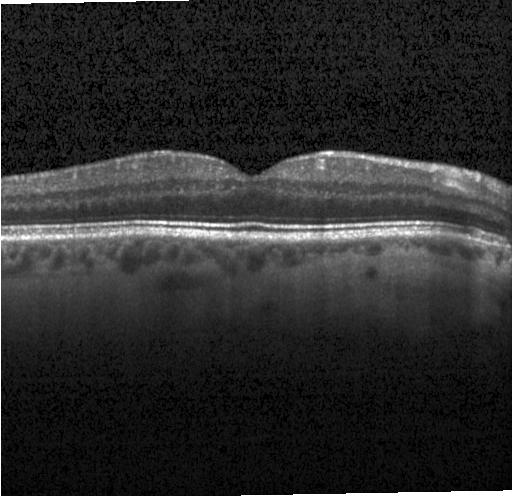

Retinal OCT cross-section showing no choroidal neovascularization, diabetic macular edema, or drusen.